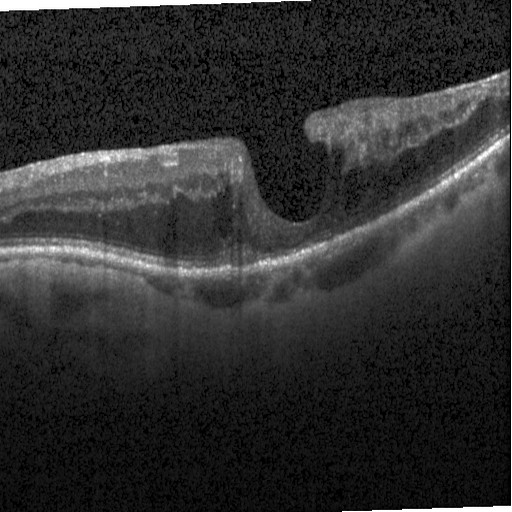 OCT scan showing diabetic macular edema (DME).